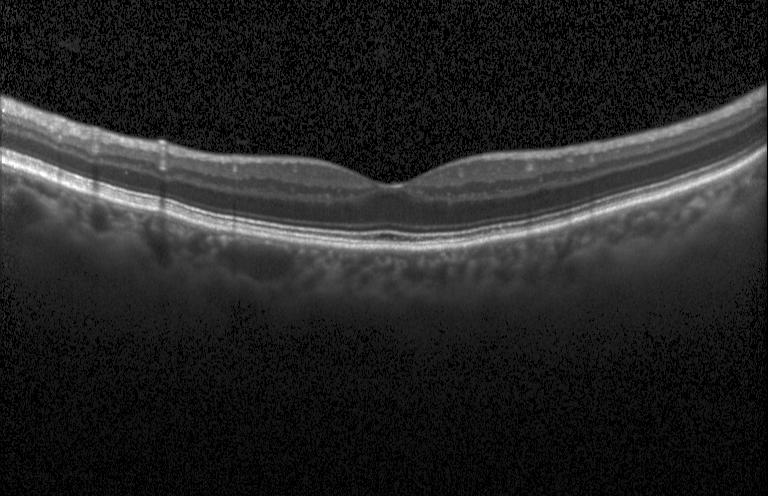 Fovea-centered · retinal OCT cross-section · SD-OCT
Finding: neither CNV, DME, nor drusen.